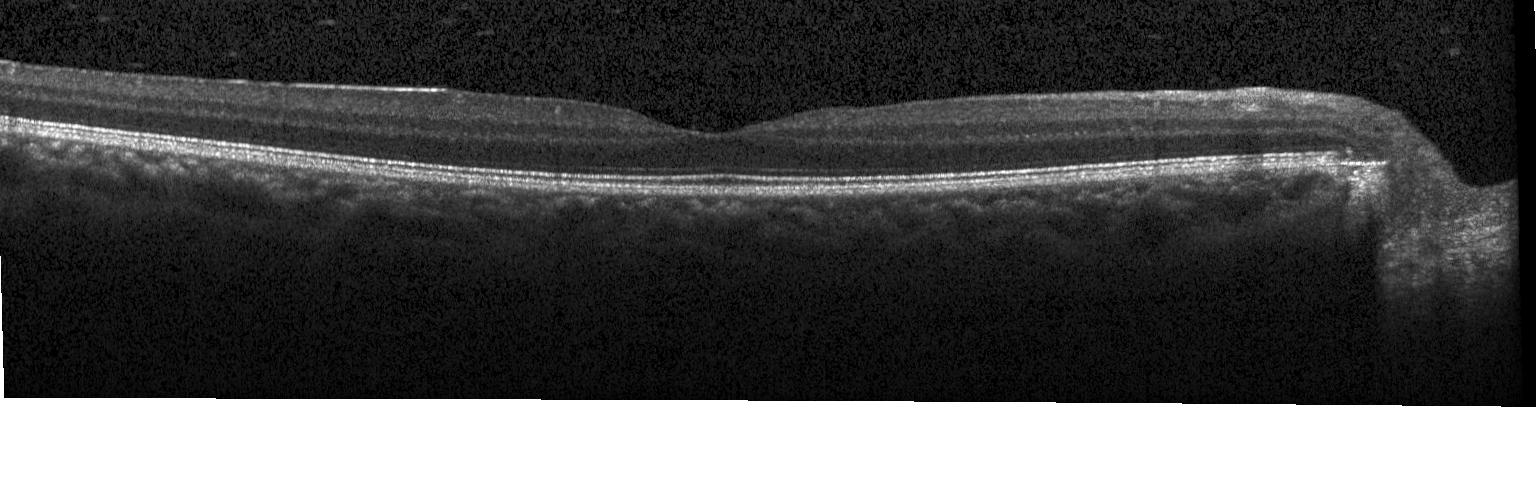
Retinal OCT B-scan · acquired on a Heidelberg Spectralis · spectral-domain optical coherence tomography · centered on the fovea.
No CNV, DME, or drusen.